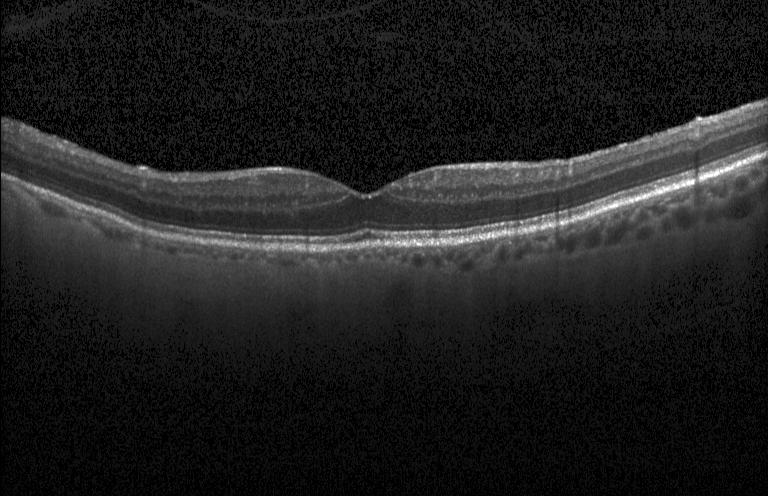 Retinal OCT B-scan
Diagnosis: no choroidal neovascularization, no diabetic macular edema, and no drusen.